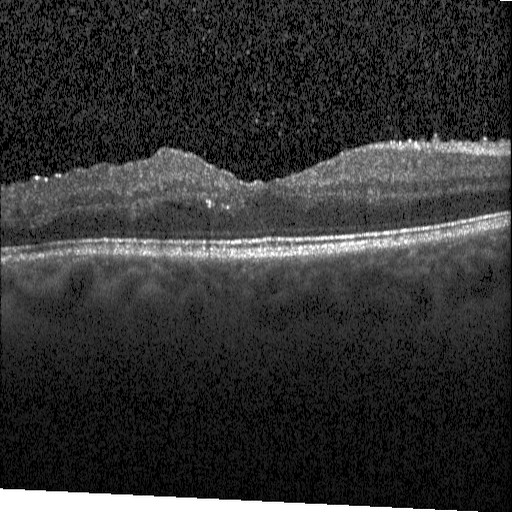

Centered on the fovea; OCT line scan.
Finding: diabetic macular edema.